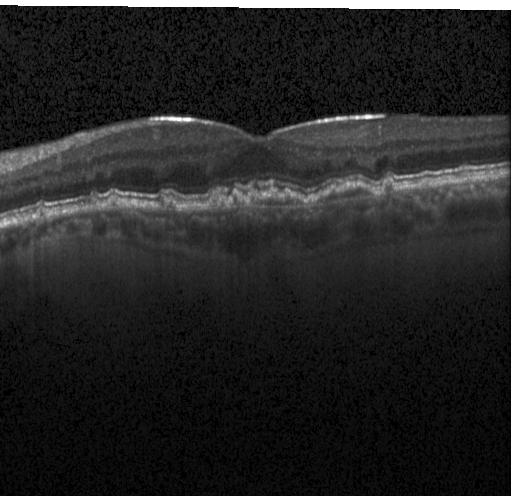 OCT B-scan; SD-OCT — Multiple drusen.